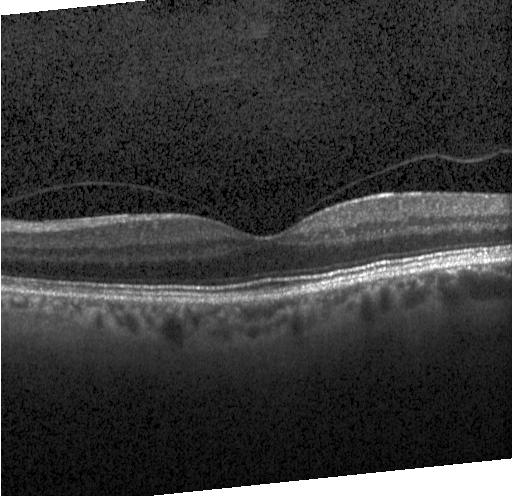
Heidelberg Spectralis OCT system · spectral-domain optical coherence tomography · OCT B-scan — Neither choroidal neovascularization, diabetic macular edema, nor drusen.